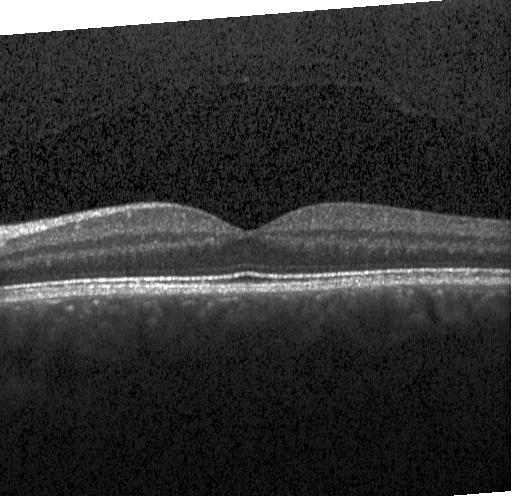

Heidelberg Spectralis; macular scan; optical coherence tomography B-scan.
Diagnosis: no evidence of choroidal neovascularization, diabetic macular edema, or drusen.